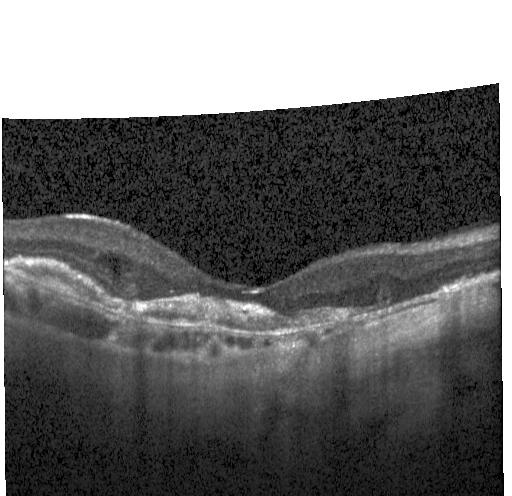
Retinal OCT cross-section.
Assessment: choroidal neovascularization (CNV).